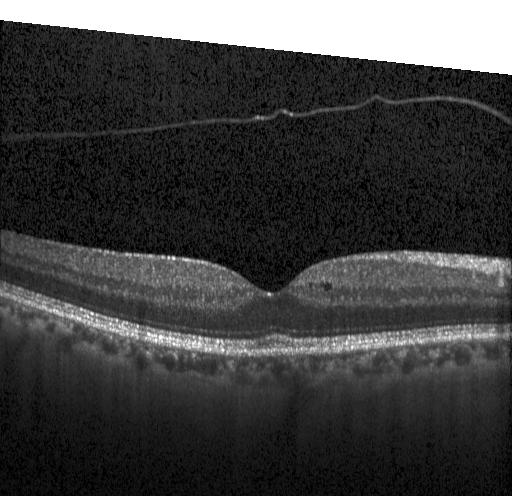 Retinal OCT B-scan
Macular OCT: diabetic macular edema (DME).